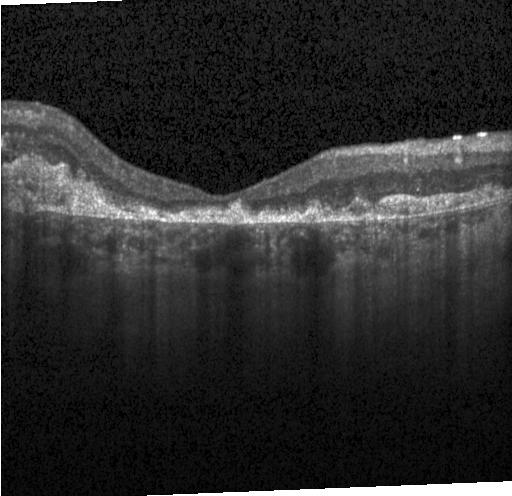 Spectral-domain optical coherence tomography, retinal OCT B-scan
Diagnosis: CNV.